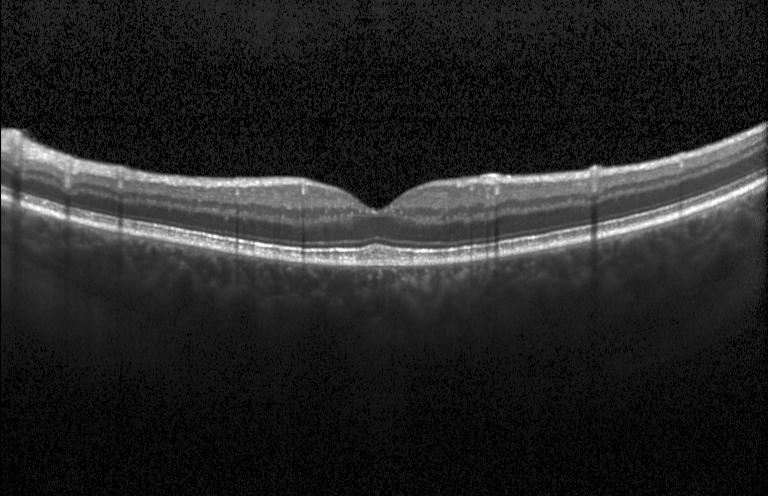
Heidelberg Spectralis · optical coherence tomography scan · through the macula.
This B-scan demonstrates neither choroidal neovascularization, diabetic macular edema, nor drusen.